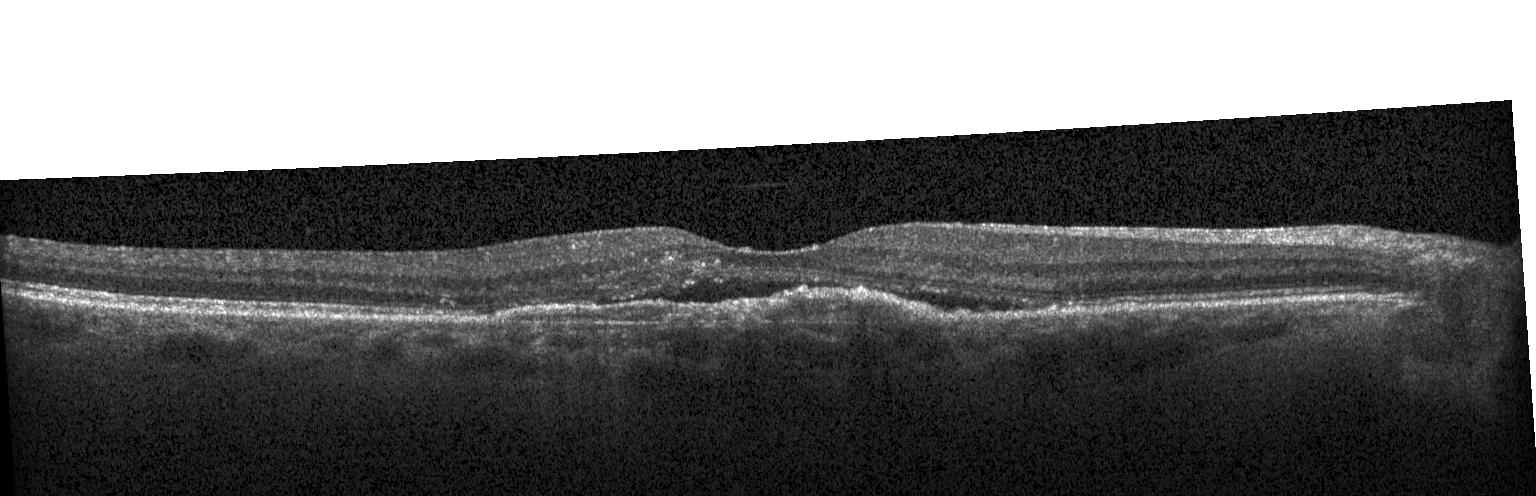 Macular OCT: choroidal neovascularization.